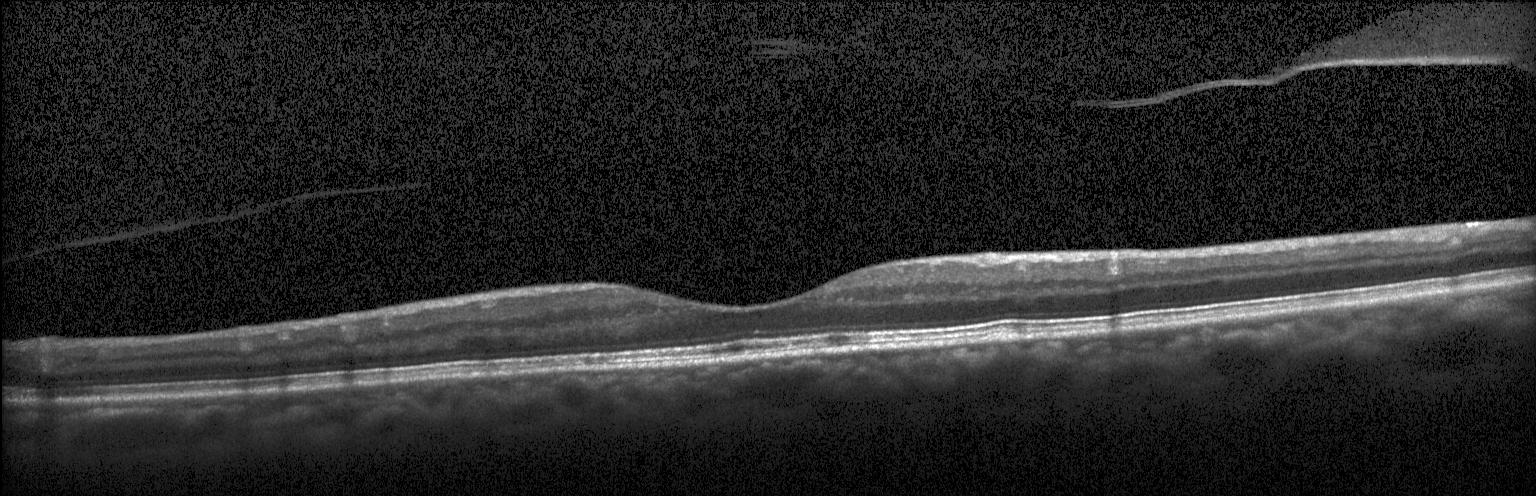

Instrument: Heidelberg Spectralis; retinal OCT cross-section; macular scan
Finding: neither CNV, DME, nor drusen.